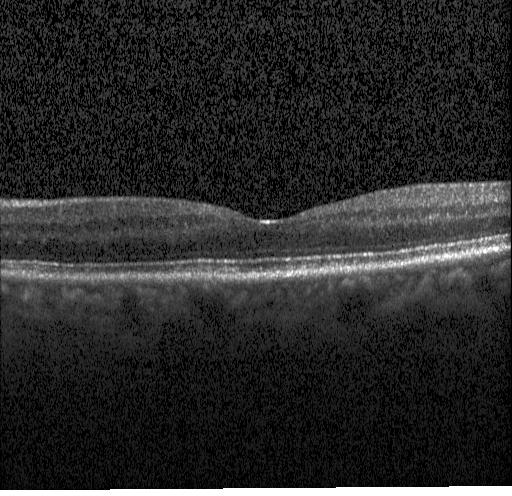

SD-OCT; optical coherence tomography scan; acquired on a Heidelberg Spectralis; centered on the fovea. Macular OCT: no choroidal neovascularization, no diabetic macular edema, and no drusen.